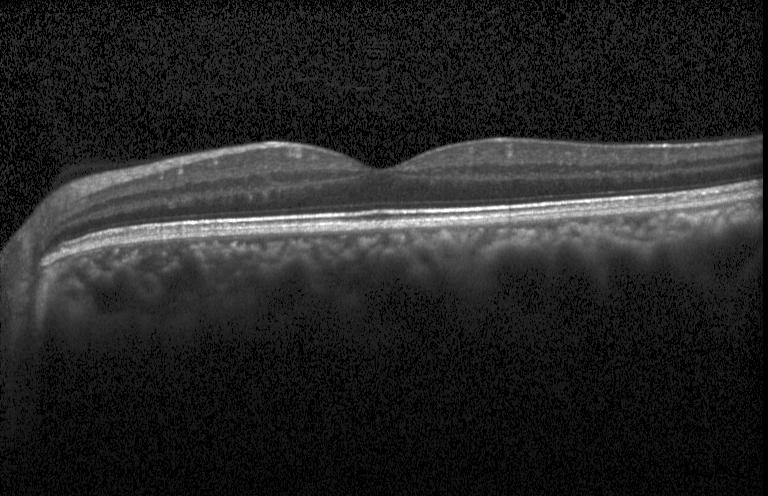
OCT scan showing neither choroidal neovascularization, diabetic macular edema, nor drusen.